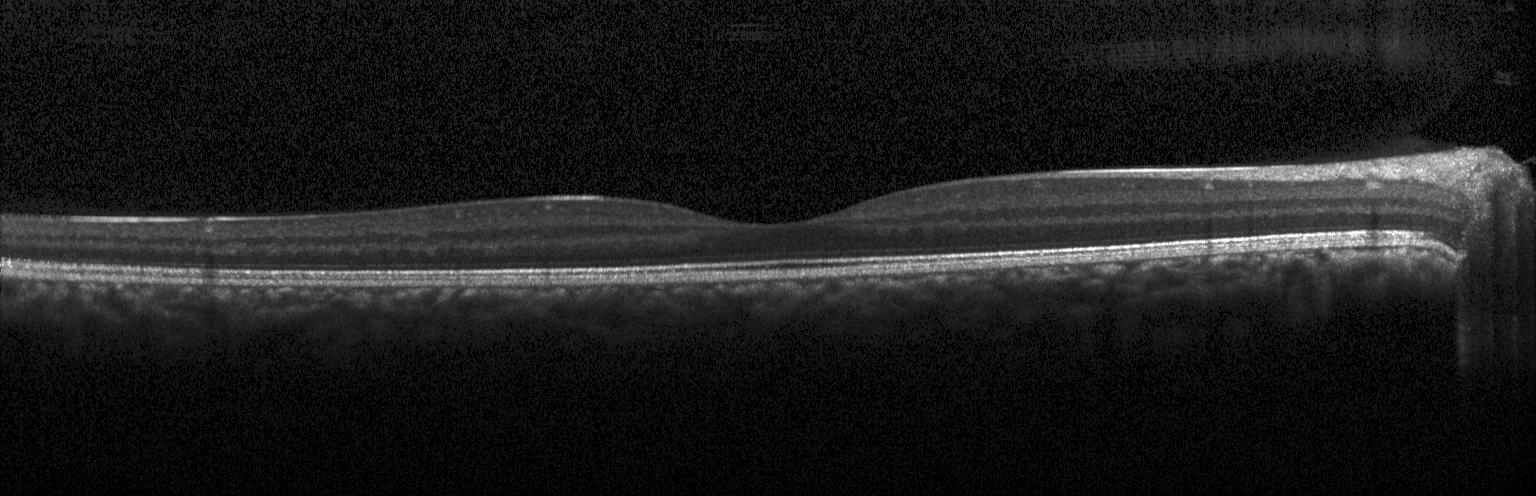 Impression: neither choroidal neovascularization, diabetic macular edema, nor drusen.